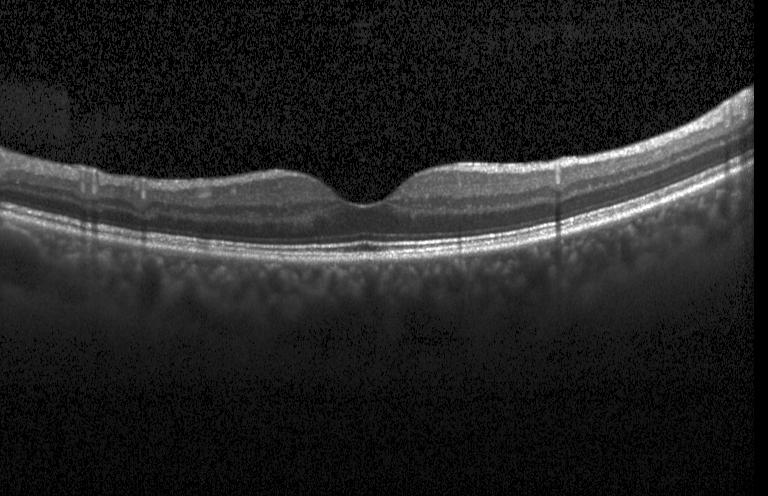

SD-OCT. Macular scan. Optical coherence tomography B-scan — No CNV, no DME, and no drusen.